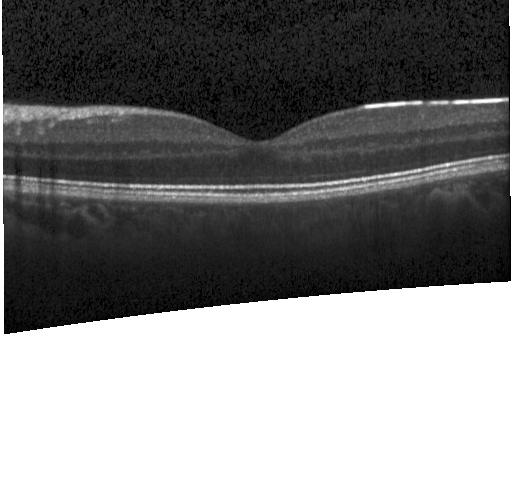

OCT B-scan showing neither choroidal neovascularization, diabetic macular edema, nor drusen.